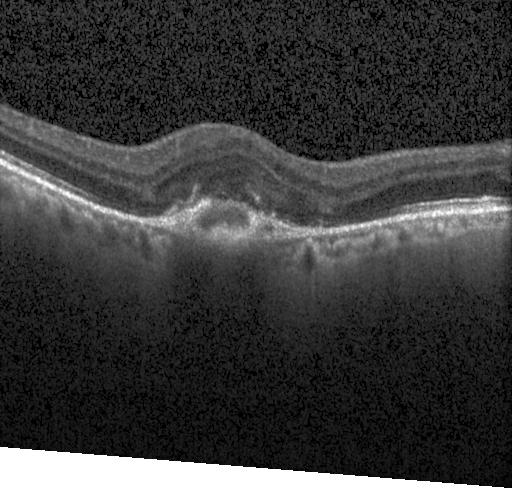

OCT B-scan, acquired on a Heidelberg Spectralis, fovea-centered, SD-OCT — Impression: choroidal neovascularization.